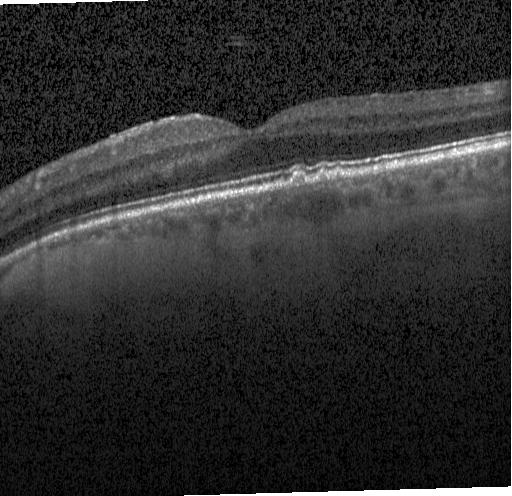
Acquired on a Heidelberg Spectralis, fovea-centered, optical coherence tomography B-scan, spectral-domain optical coherence tomography
Finding: sub-RPE drusenoid deposits.